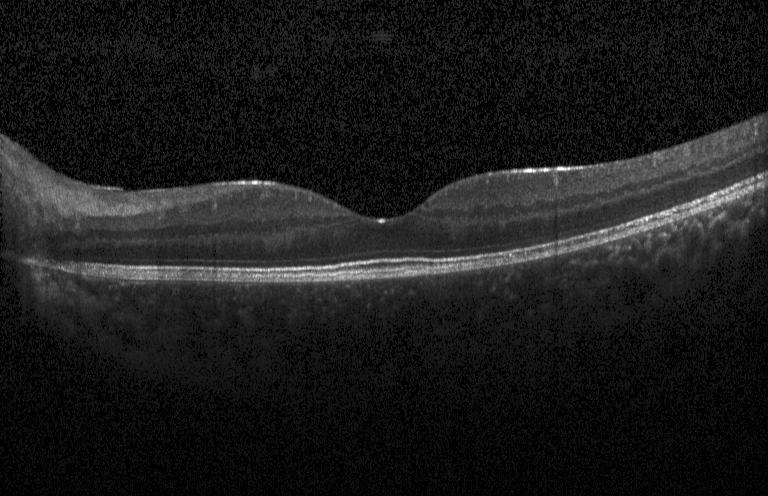
OCT line scan
Finding: no choroidal neovascularization, diabetic macular edema, or drusen.